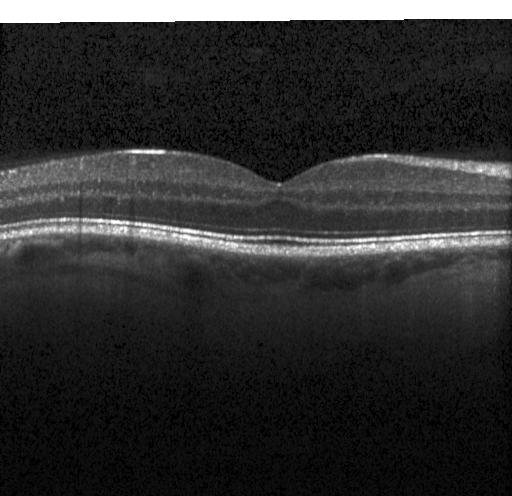 Assessment: no evidence of CNV, DME, or drusen.